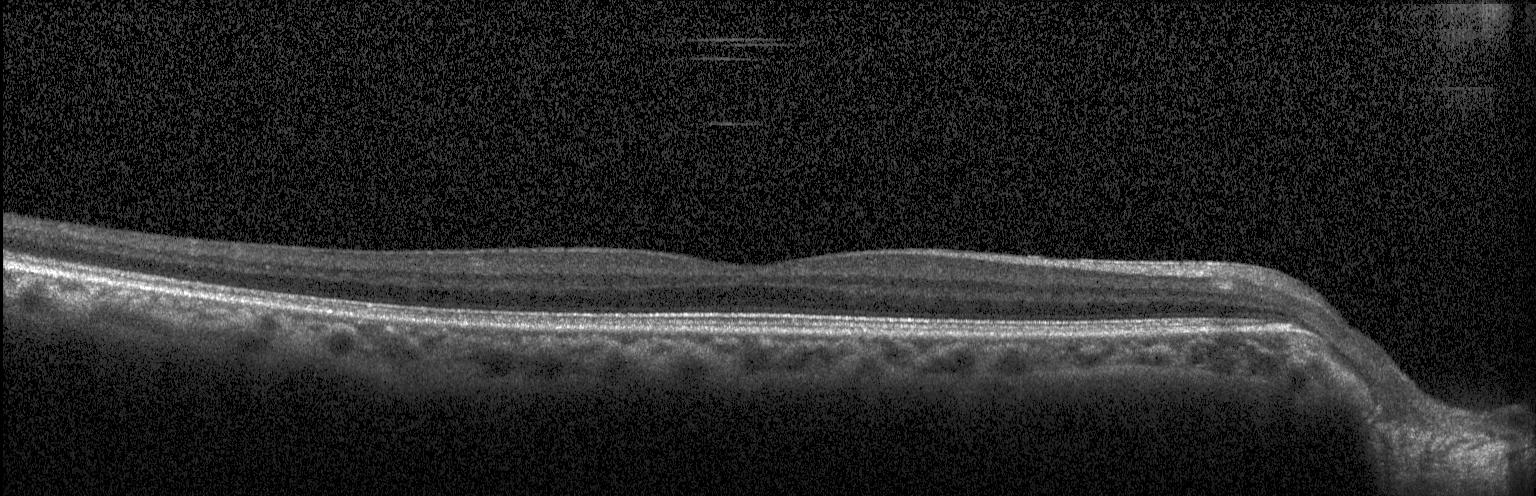
Diagnosis: no evidence of CNV, DME, or drusen.